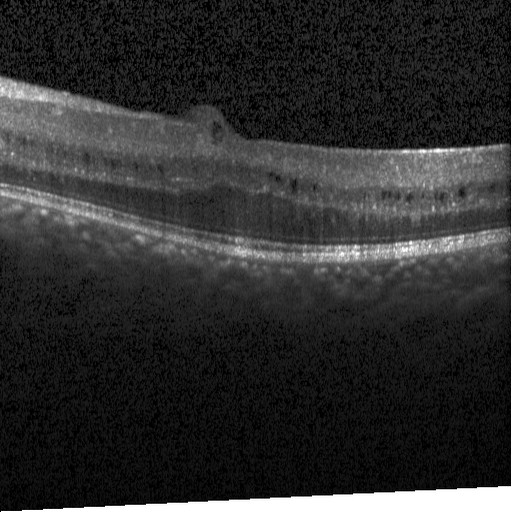
Centered on the fovea · optical coherence tomography B-scan · spectral-domain optical coherence tomography · Heidelberg Spectralis.
OCT finding: diabetic macular edema.